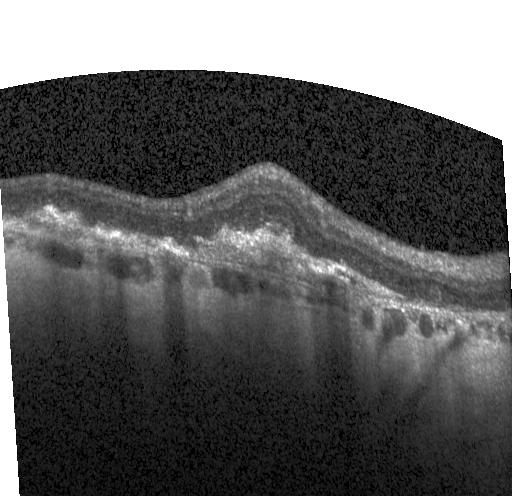 Diagnosis: a choroidal neovascular membrane.